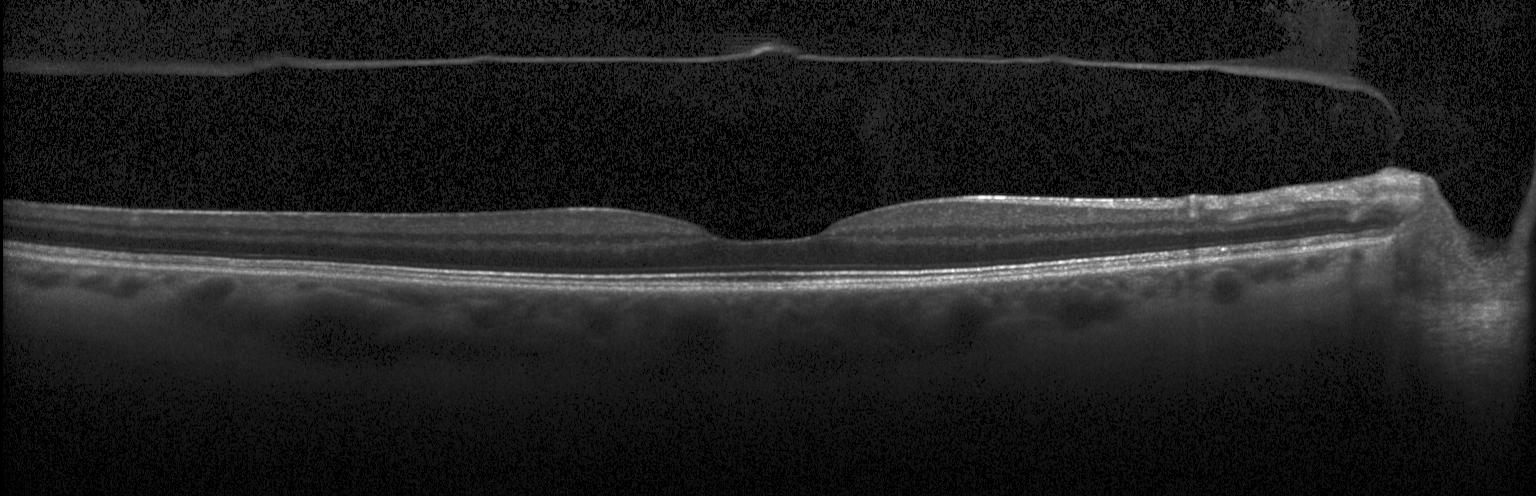 Acquired on a Heidelberg Spectralis · retinal OCT cross-section · fovea-centered · spectral-domain OCT
No choroidal neovascularization, diabetic macular edema, or drusen.